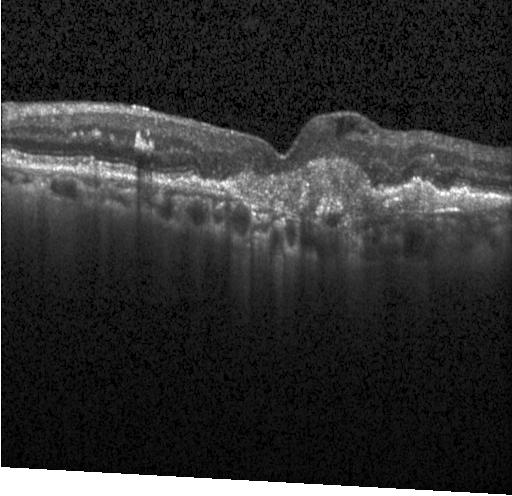 OCT line scan; acquired on a Heidelberg Spectralis
Finding: choroidal neovascularization (CNV).